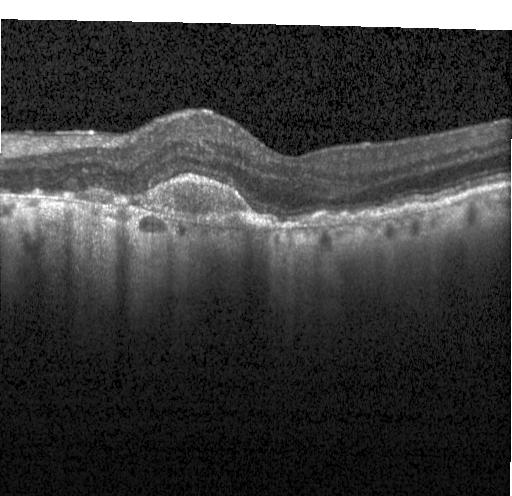

Retinal OCT B-scan — Impression: choroidal neovascularization.